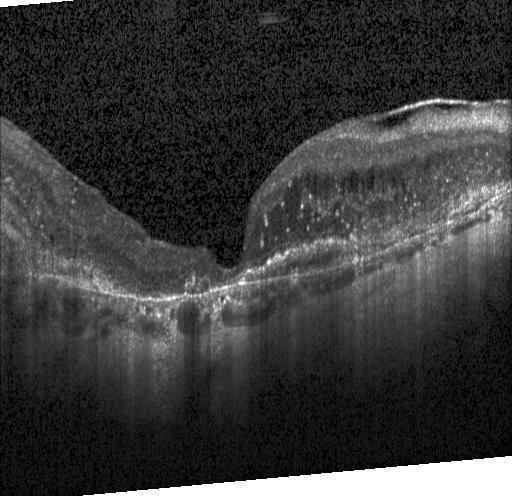
Impression: choroidal neovascularization.